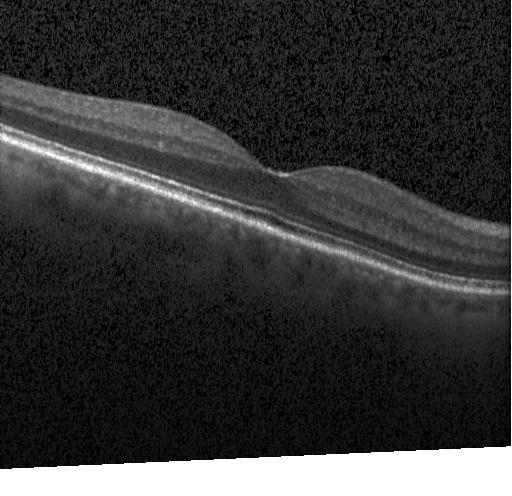

Retinal OCT B-scan, through the macula — Diagnosis: no evidence of choroidal neovascularization, diabetic macular edema, or drusen.